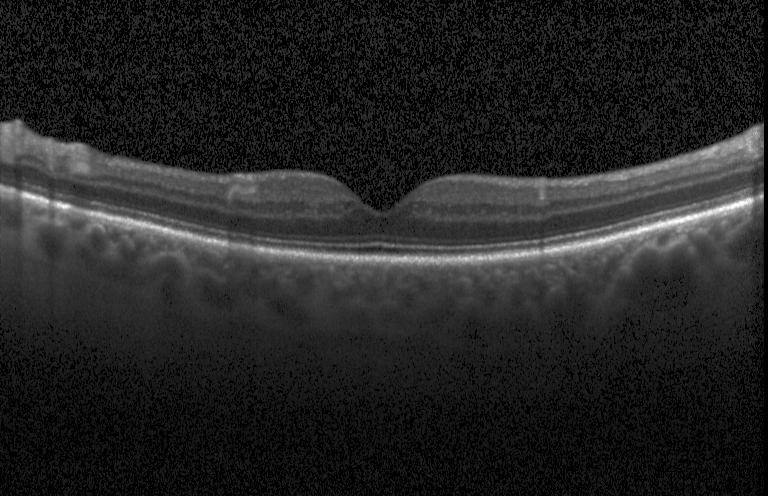
Spectral-domain optical coherence tomography · instrument: Heidelberg Spectralis · OCT B-scan · centered on the fovea.
Diagnosis: neither choroidal neovascularization, diabetic macular edema, nor drusen.